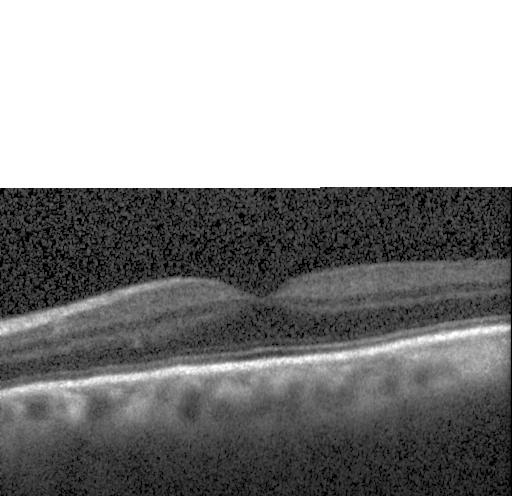
Retinal OCT B-scan.
Impression: neither CNV, DME, nor drusen.